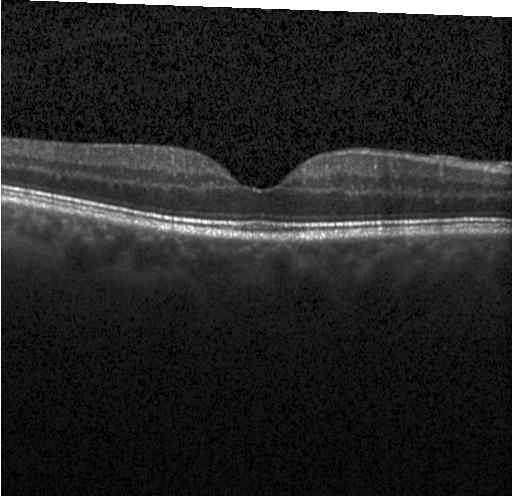
Assessment: no choroidal neovascularization, no diabetic macular edema, and no drusen.